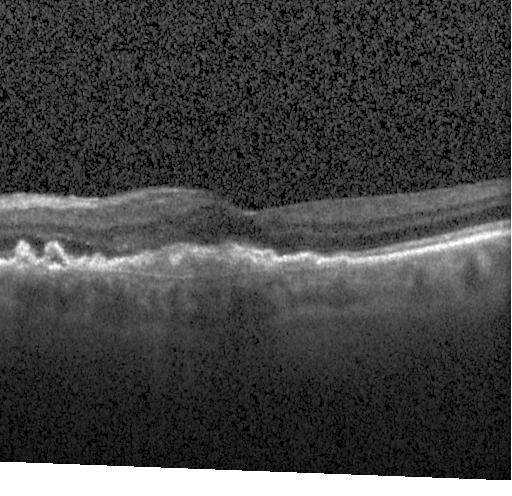
Choroidal neovascularization (CNV).